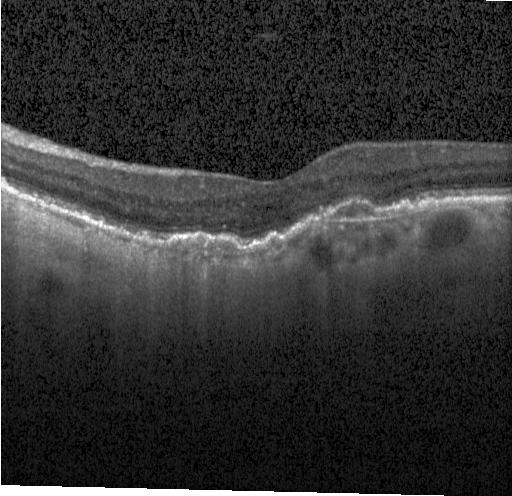
Impression: choroidal neovascularization.